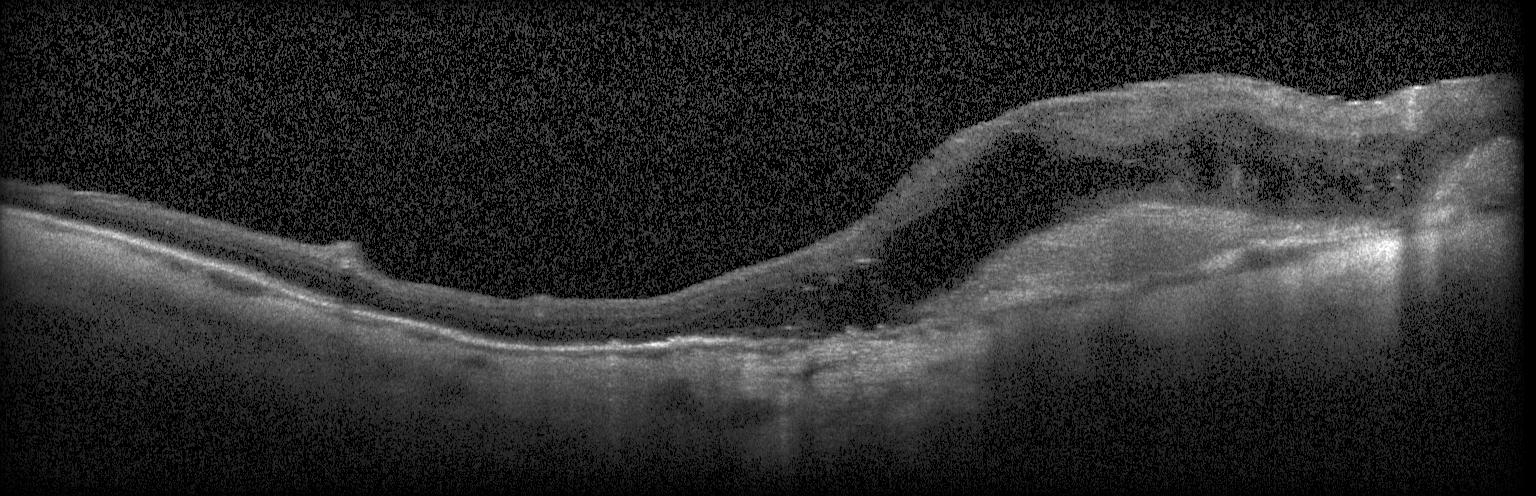
Spectral-domain optical coherence tomography, acquired on a Heidelberg Spectralis, optical coherence tomography B-scan.
The scan shows a choroidal neovascular membrane.